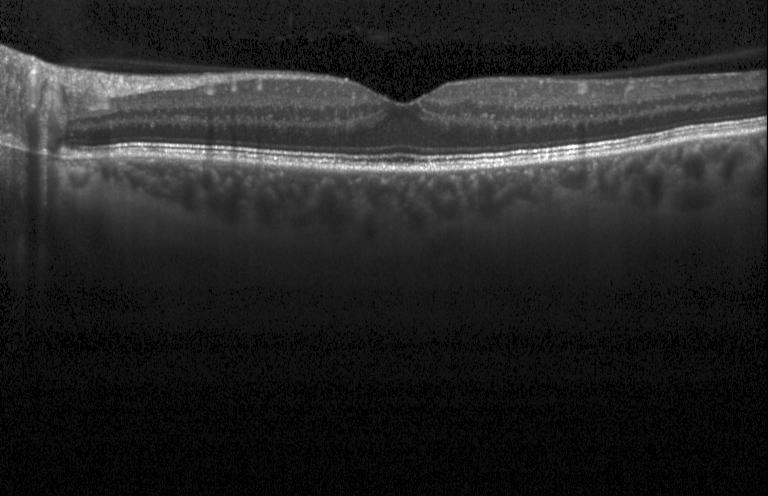 Instrument: Heidelberg Spectralis; optical coherence tomography B-scan; centered on the fovea; SD-OCT
OCT finding: no evidence of CNV, DME, or drusen.